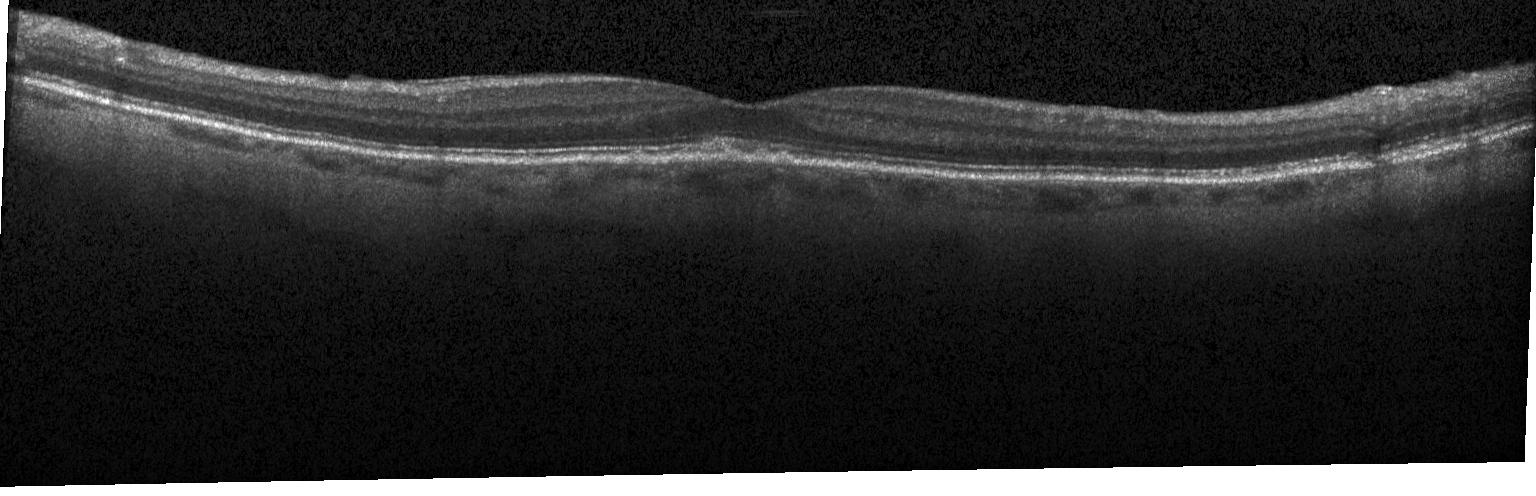 Retinal OCT cross-section showing sub-RPE drusenoid deposits.